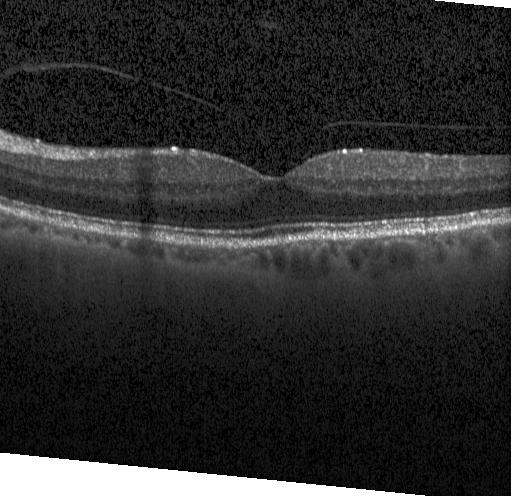
Macular OCT: no evidence of choroidal neovascularization, diabetic macular edema, or drusen.